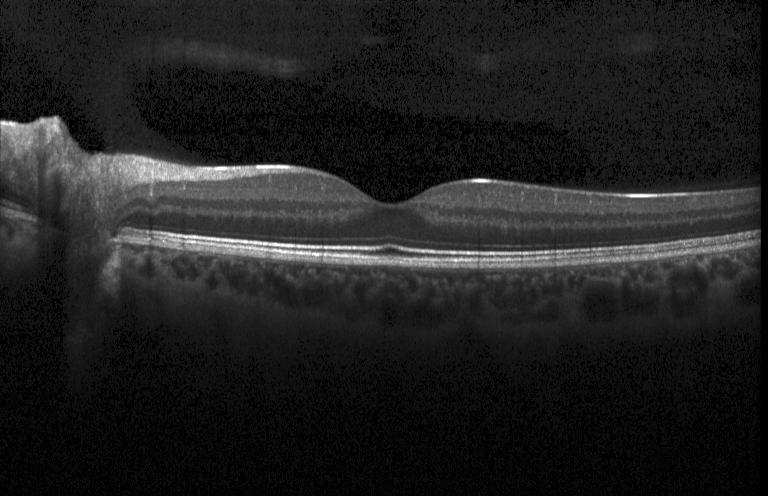
Retinal OCT B-scan · spectral-domain OCT · through the macula
The scan shows no choroidal neovascularization, diabetic macular edema, or drusen.